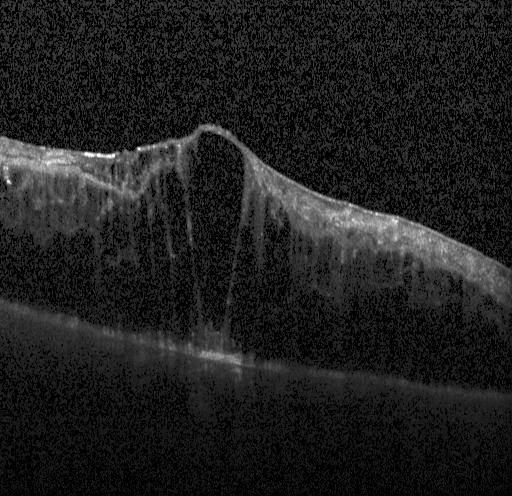 OCT B-scan; spectral-domain optical coherence tomography. Finding: DME.